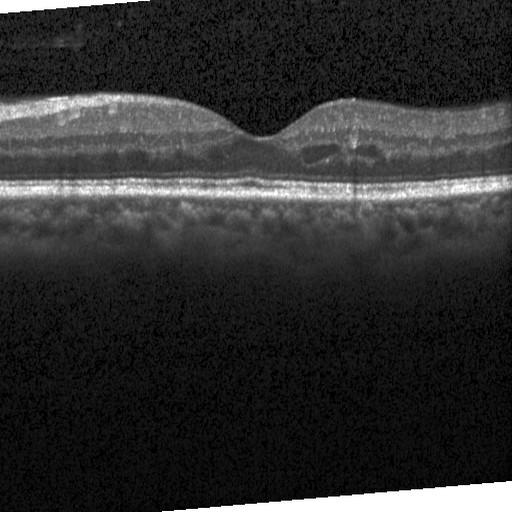

Horizontal scan through the fovea; spectral-domain optical coherence tomography; Heidelberg Spectralis OCT system; OCT line scan — Assessment: diabetic macular edema.